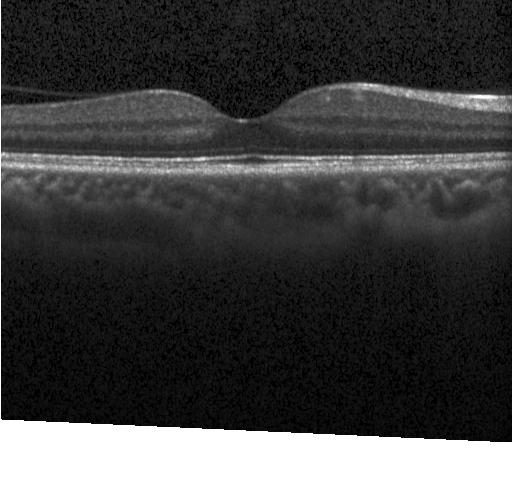 Finding: no choroidal neovascularization, diabetic macular edema, or drusen.